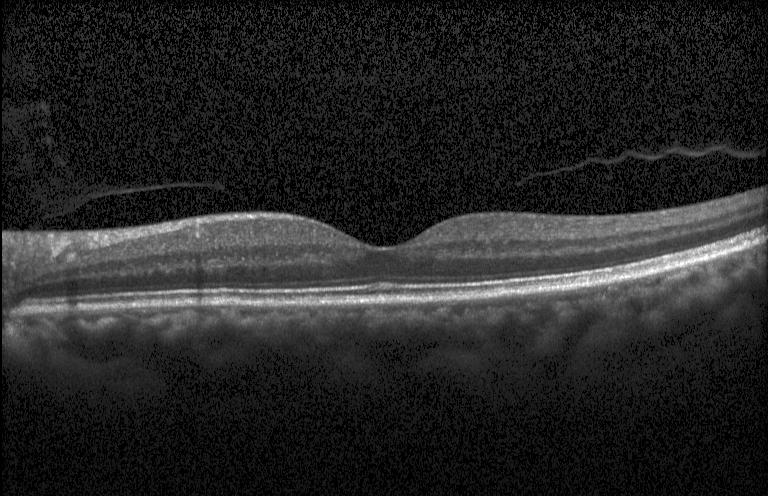 Through the macula; Heidelberg Spectralis OCT system; spectral-domain OCT; OCT line scan — Diagnosis: no evidence of choroidal neovascularization, diabetic macular edema, or drusen.